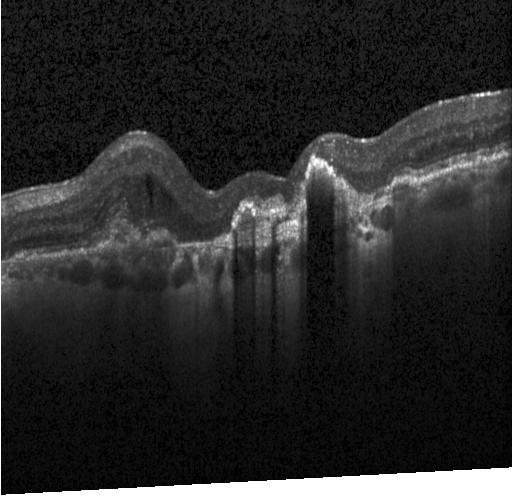

Optical coherence tomography B-scan.
This B-scan demonstrates choroidal neovascularization.